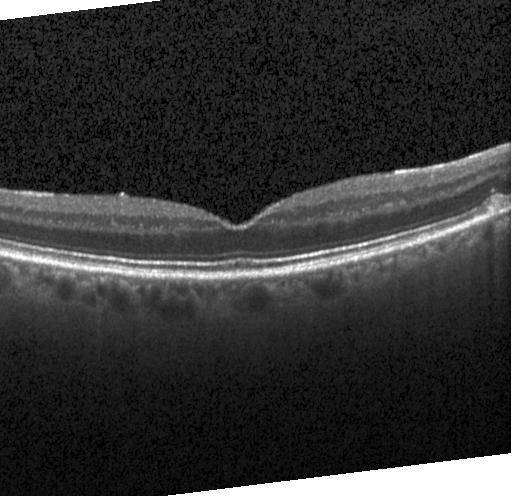 Macular OCT demonstrating neither CNV, DME, nor drusen.